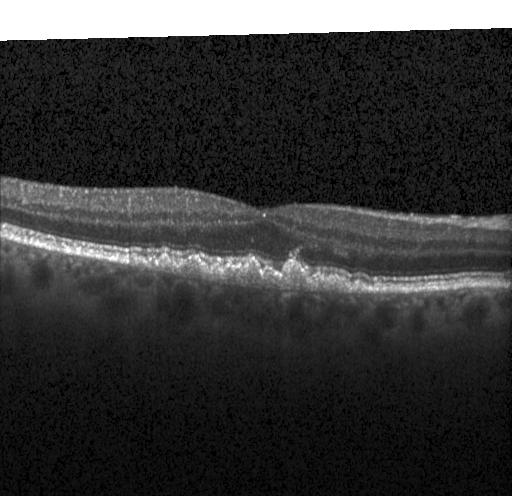
OCT B-scan · Heidelberg Spectralis OCT system — The scan shows drusen.